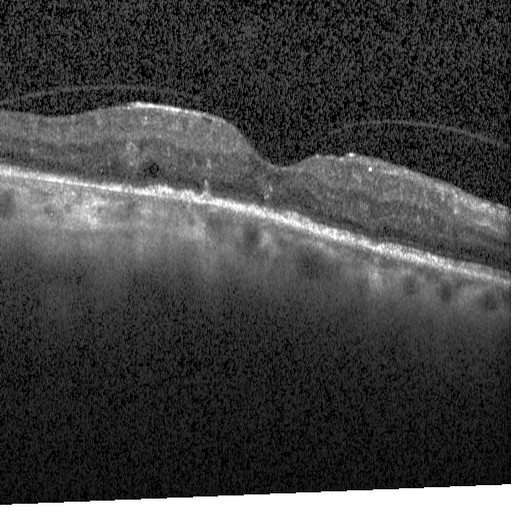 Retinal OCT cross-section showing DME.